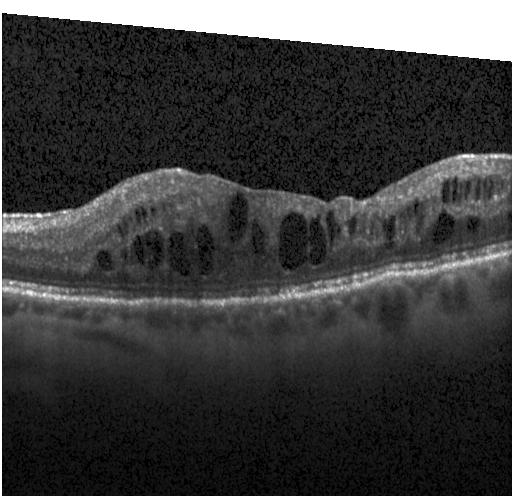

OCT B-scan — Impression: diabetic macular edema (DME).